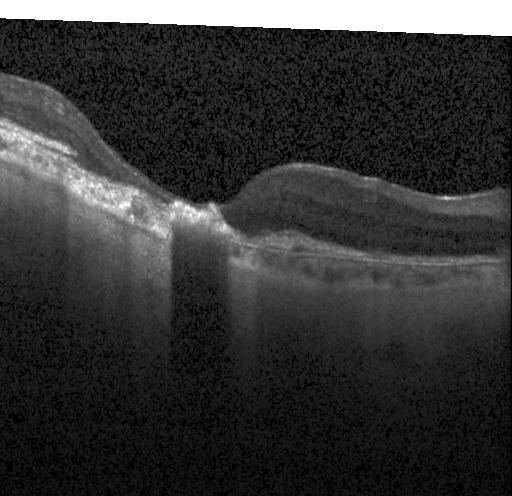
OCT B-scan showing choroidal neovascularization.